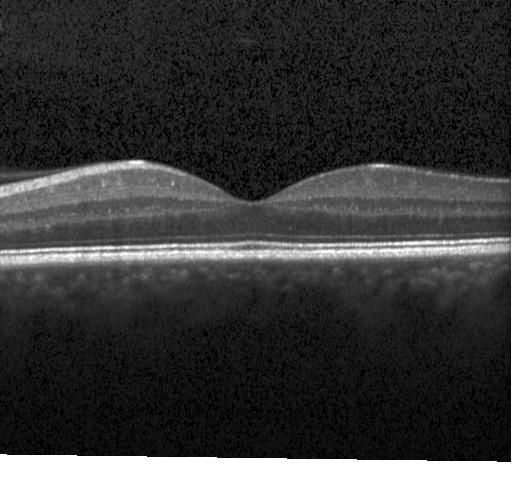
Optical coherence tomography B-scan. Impression: no choroidal neovascularization, no diabetic macular edema, and no drusen.